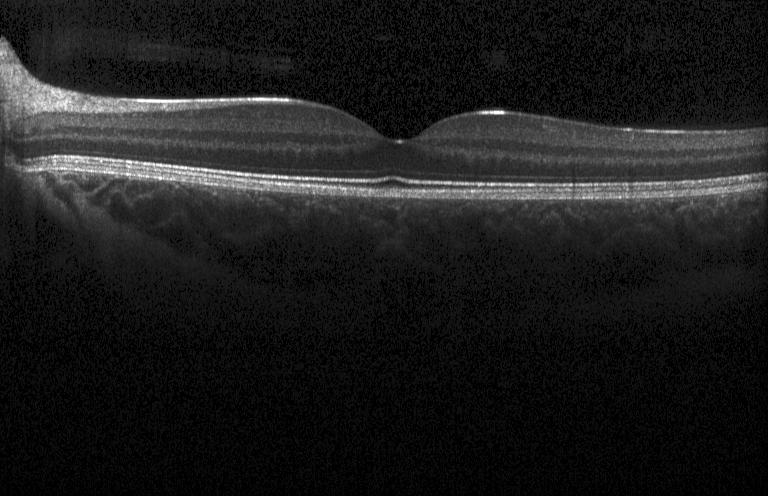

Impression: no evidence of choroidal neovascularization, diabetic macular edema, or drusen.